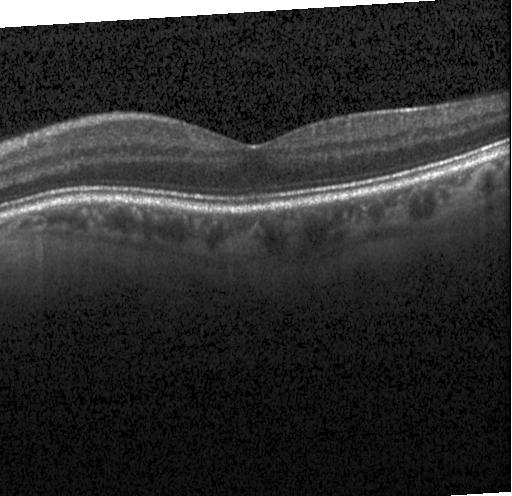

Finding: neither CNV, DME, nor drusen.